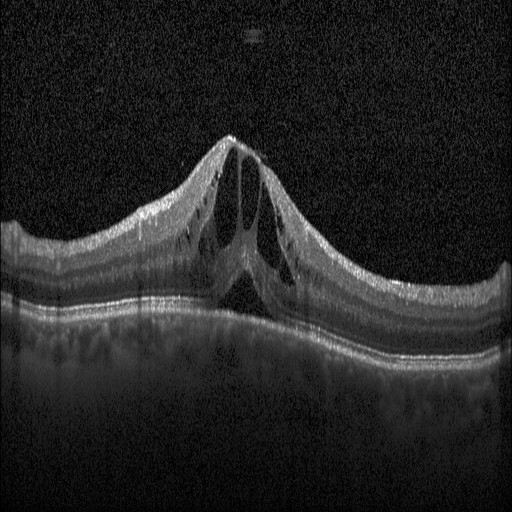

Instrument: Heidelberg Spectralis; spectral-domain optical coherence tomography; optical coherence tomography B-scan.
Macular OCT: diabetic macular edema (DME).